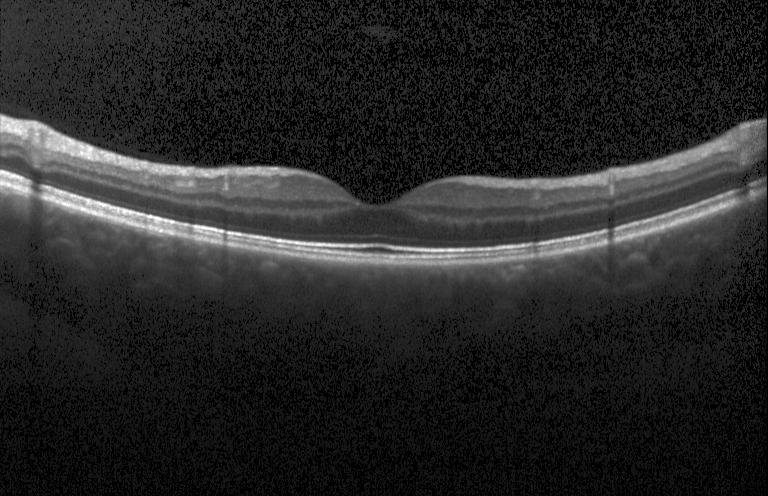

Centered on the fovea; optical coherence tomography scan; instrument: Heidelberg Spectralis; spectral-domain optical coherence tomography.
The scan shows neither choroidal neovascularization, diabetic macular edema, nor drusen.